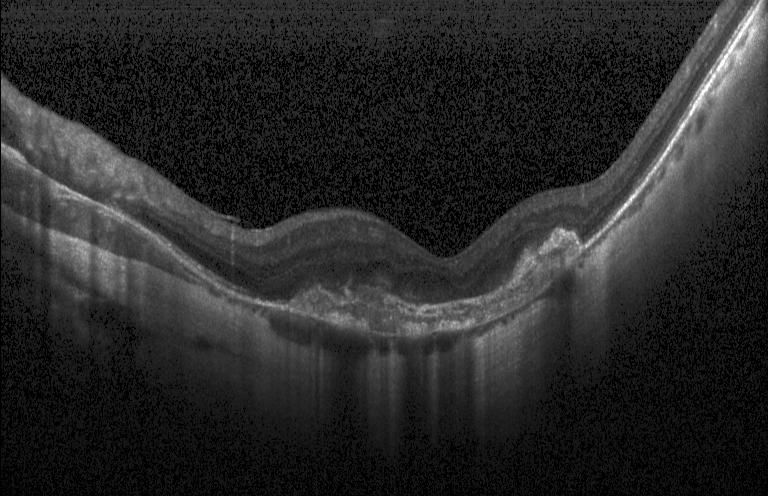
Impression: choroidal neovascularization.